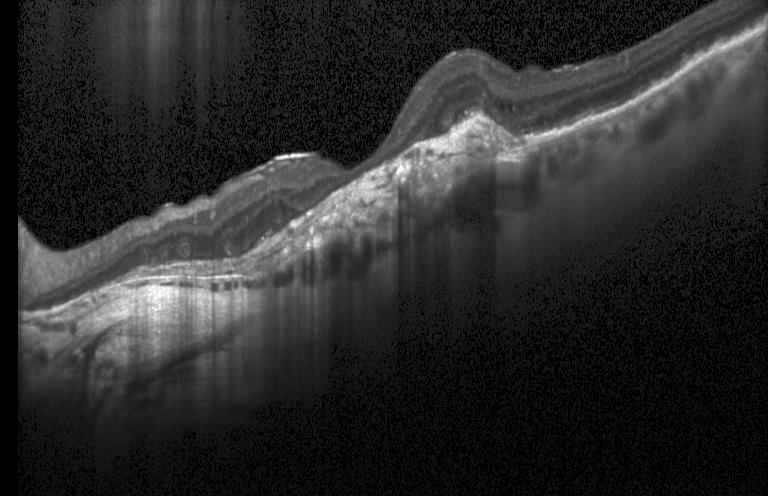 Macular OCT demonstrating choroidal neovascularization.